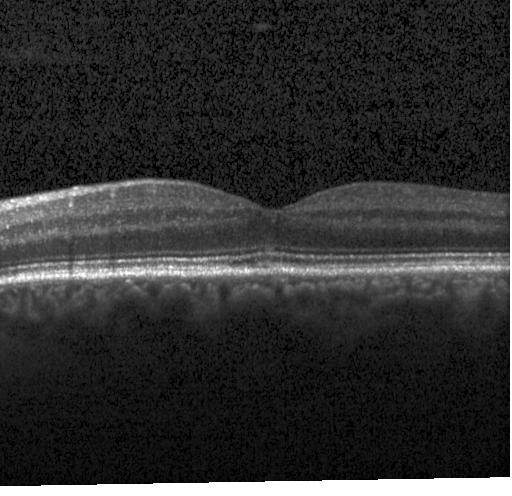 Assessment: no evidence of CNV, DME, or drusen.